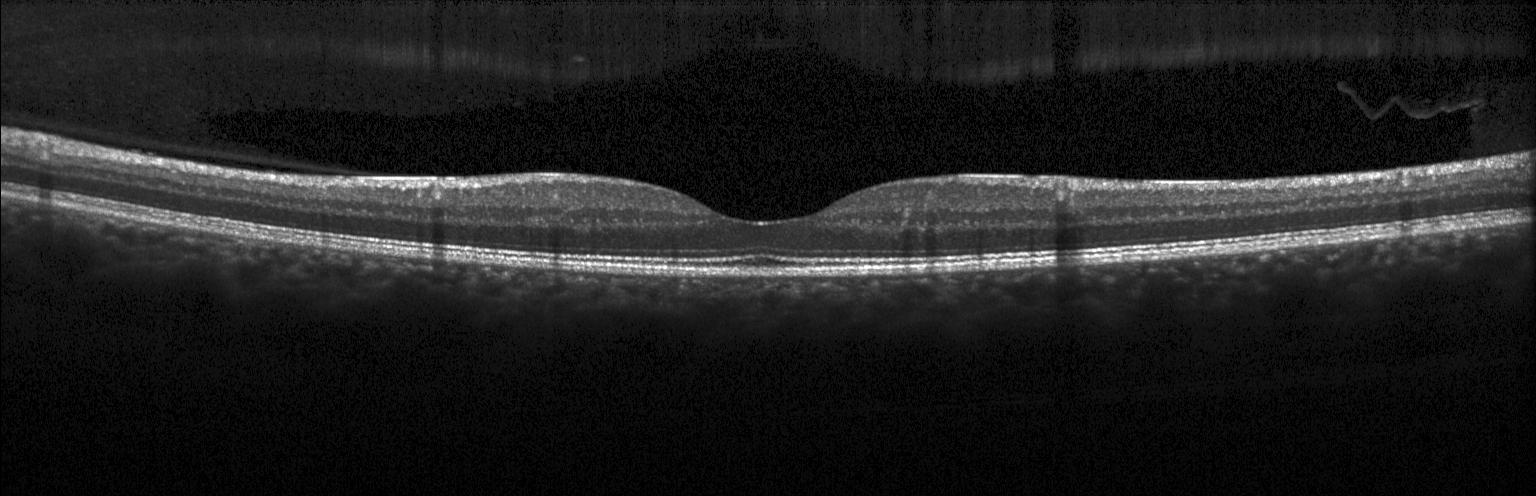

Optical coherence tomography scan. Fovea-centered. Spectral-domain OCT
Dx: no choroidal neovascularization, diabetic macular edema, or drusen.